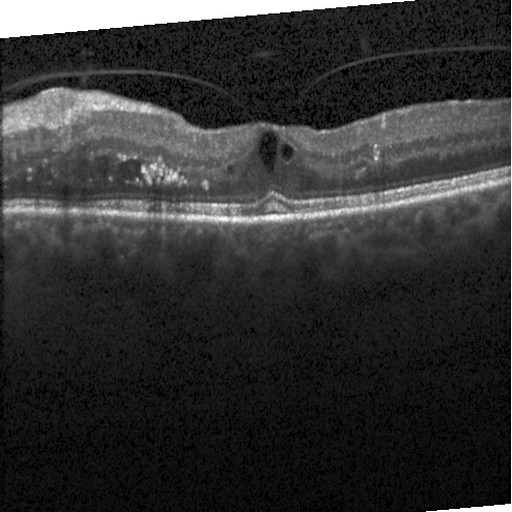
Impression: diabetic macular edema.